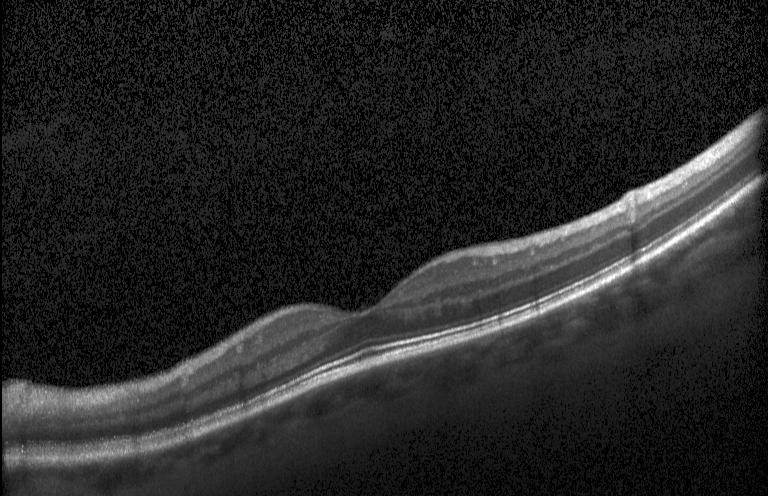
Retinal OCT cross-section showing no choroidal neovascularization, diabetic macular edema, or drusen.